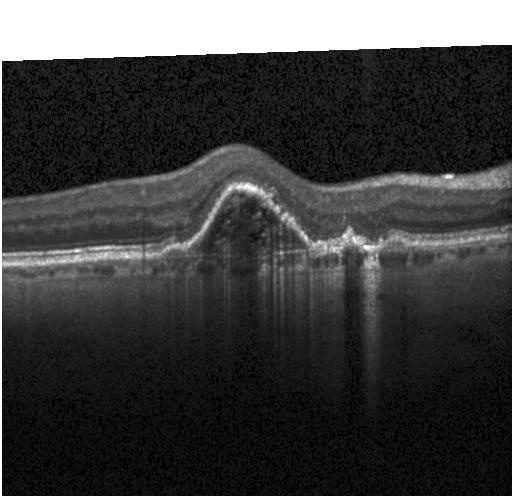

OCT finding: CNV.